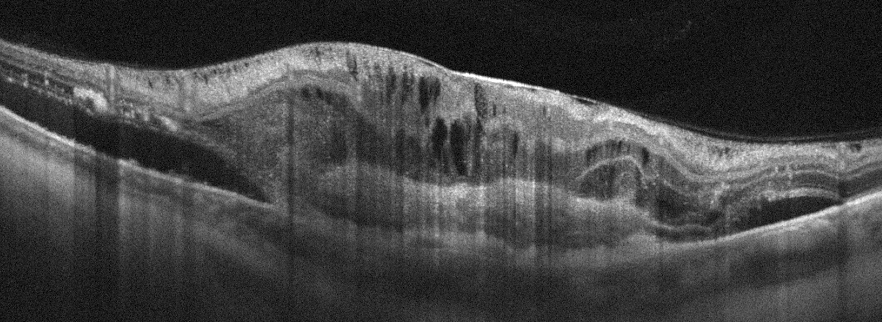
Macular OCT demonstrating age-related macular degeneration (AMD).